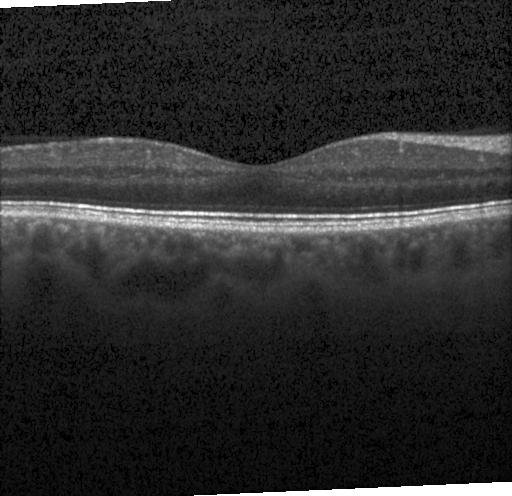 Optical coherence tomography scan
OCT finding: no CNV, no DME, and no drusen.